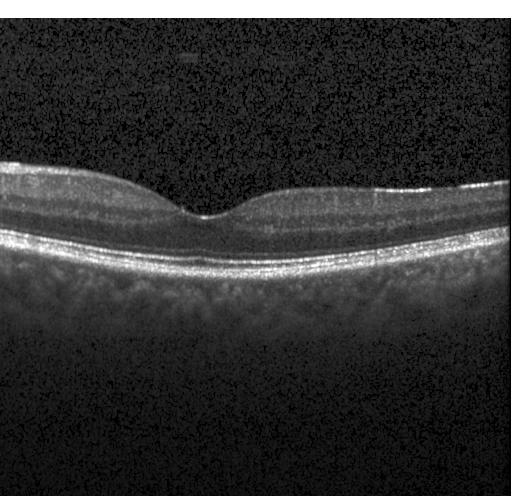 Heidelberg Spectralis · optical coherence tomography scan · spectral-domain optical coherence tomography. This B-scan demonstrates no choroidal neovascularization, diabetic macular edema, or drusen.